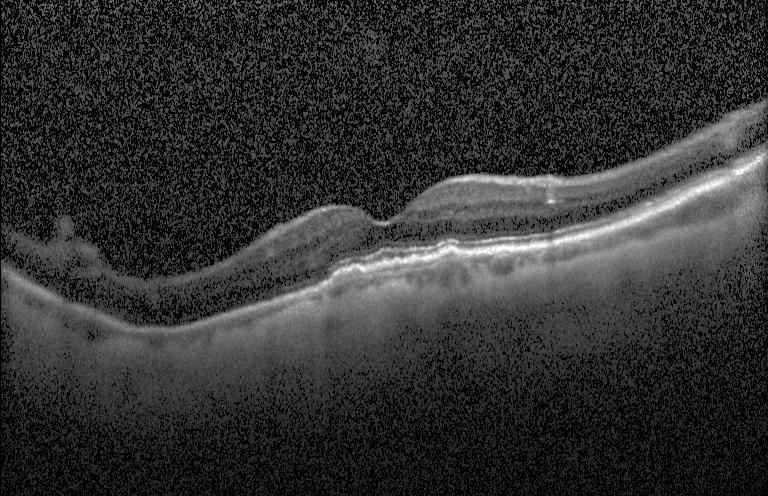 OCT B-scan.
Diagnosis: CNV.